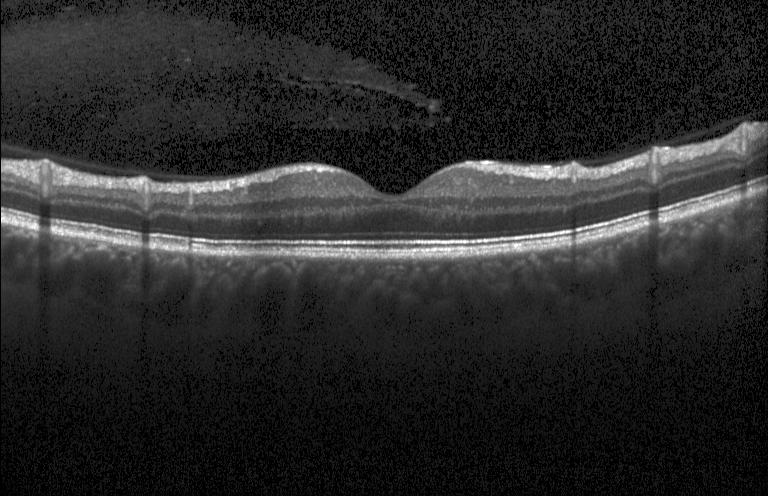
Acquired on a Heidelberg Spectralis; retinal OCT B-scan; macular scan — OCT finding: neither CNV, DME, nor drusen.